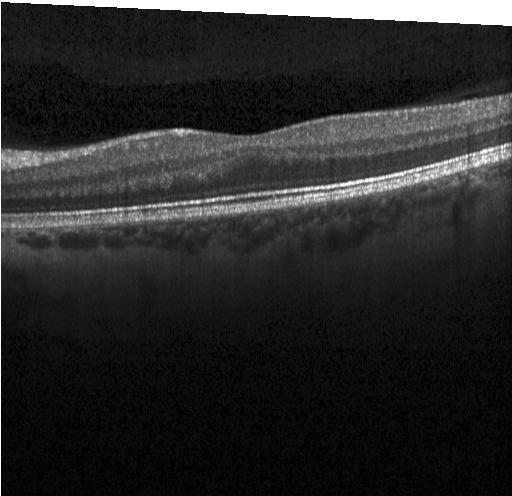

Retinal OCT B-scan.
Finding: no choroidal neovascularization, diabetic macular edema, or drusen.